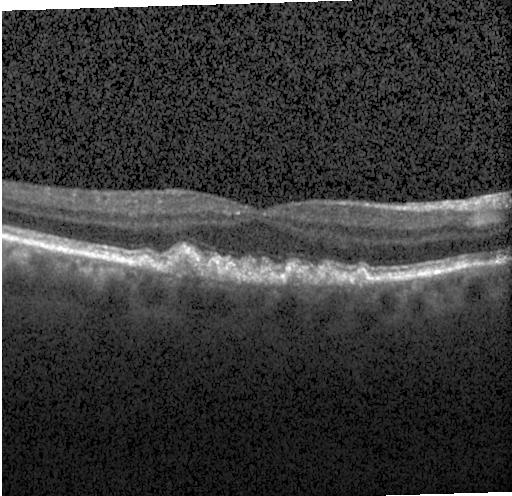
OCT line scan.
Assessment: sub-RPE drusenoid deposits.